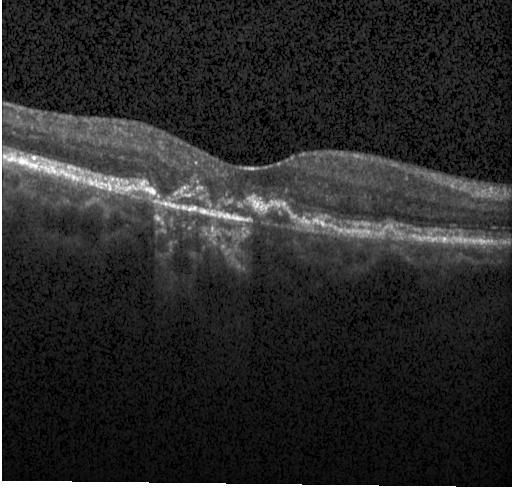
A choroidal neovascular membrane.